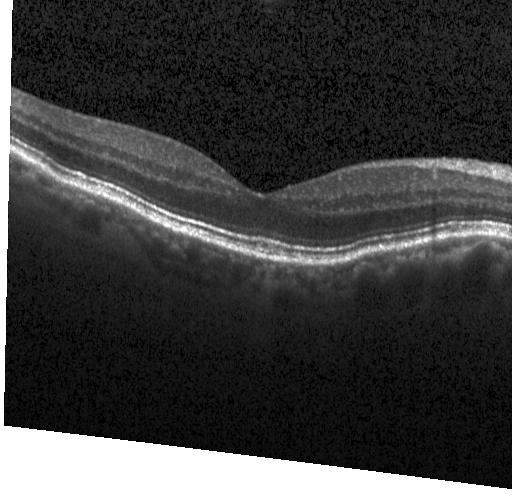 Spectral-domain optical coherence tomography · optical coherence tomography B-scan
OCT finding: no choroidal neovascularization, no diabetic macular edema, and no drusen.